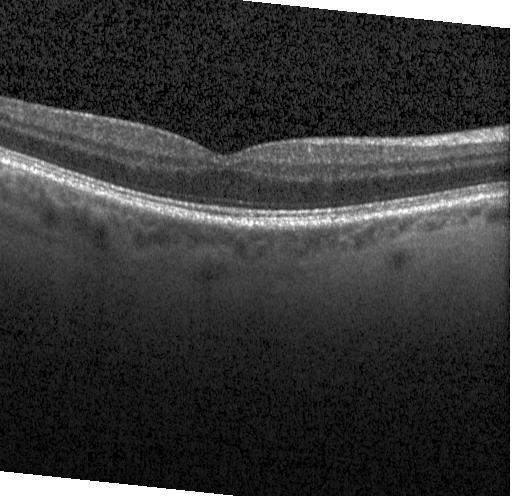 Impression: no choroidal neovascularization, diabetic macular edema, or drusen.